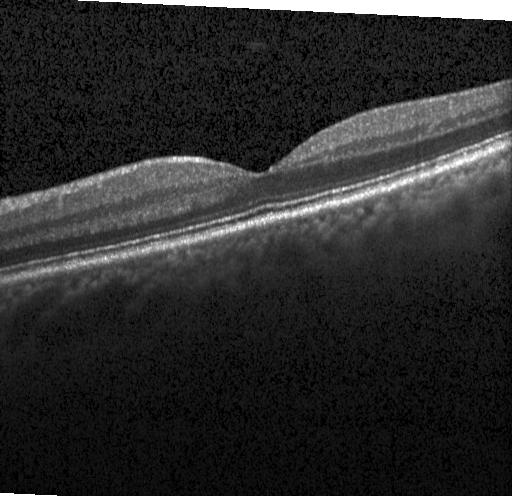 Spectral-domain OCT · optical coherence tomography B-scan · acquired on a Heidelberg Spectralis
Dx: no evidence of choroidal neovascularization, diabetic macular edema, or drusen.